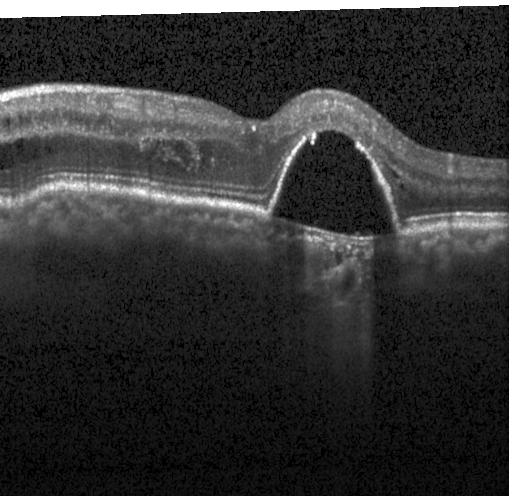

Finding: CNV.